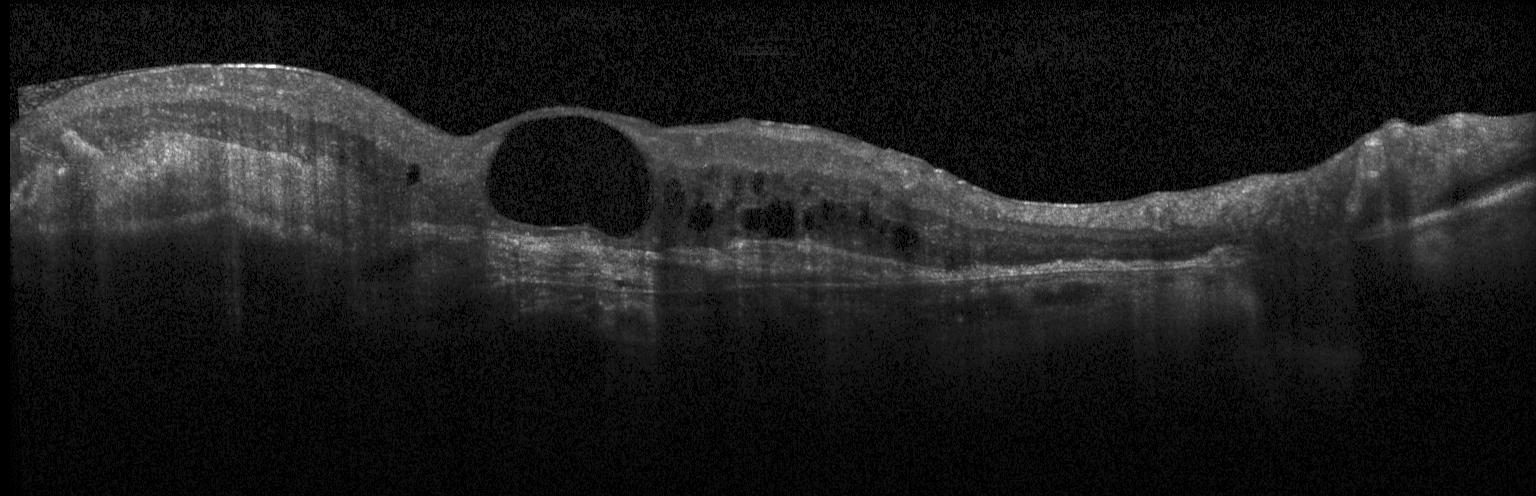
OCT B-scan · Heidelberg Spectralis · horizontal scan through the fovea · SD-OCT
Impression: choroidal neovascularization.